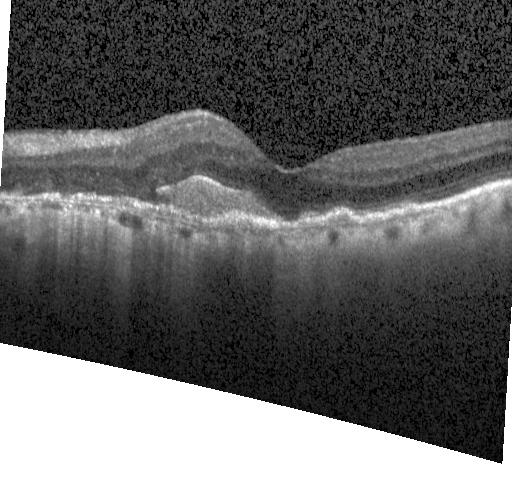

OCT B-scan. Impression: a choroidal neovascular membrane.